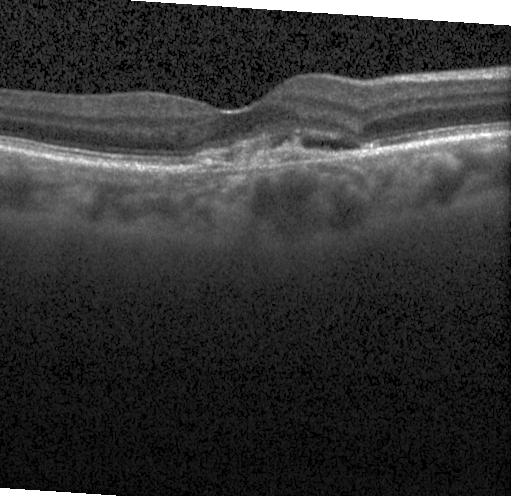

OCT line scan
Impression: a choroidal neovascular membrane.